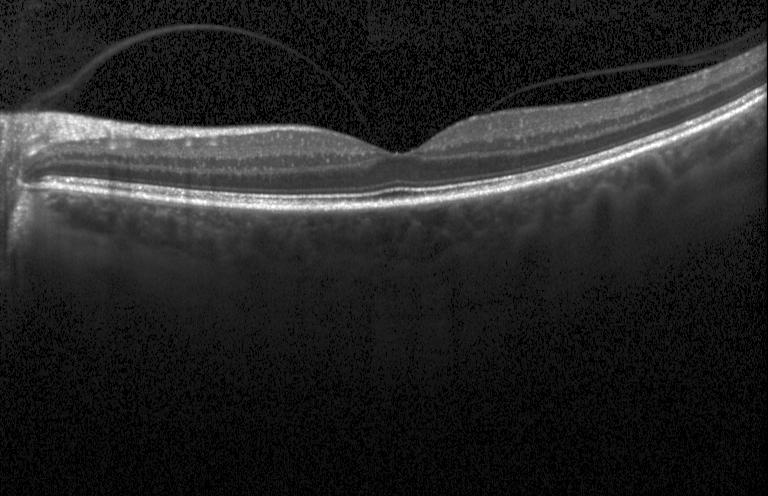

OCT line scan. No choroidal neovascularization, no diabetic macular edema, and no drusen.